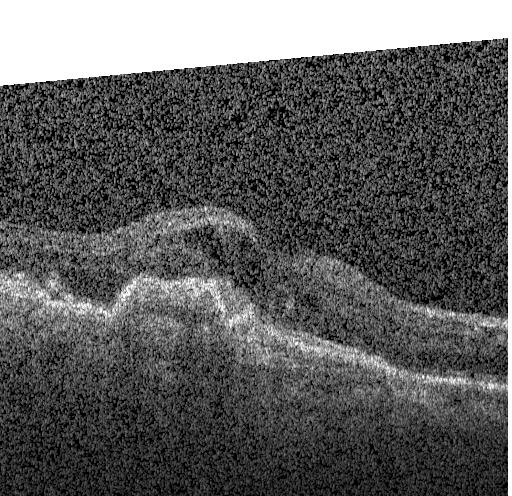 Dx: choroidal neovascularization.